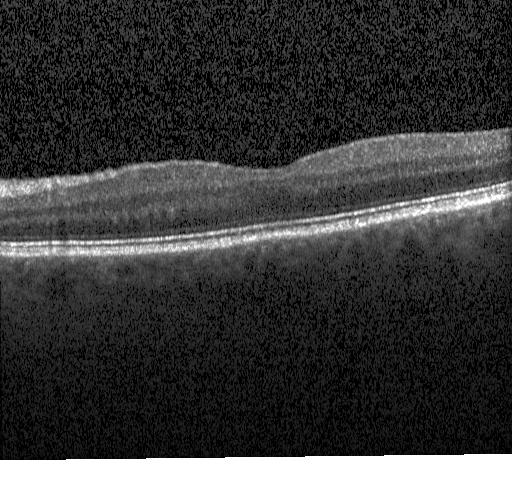
Assessment: no choroidal neovascularization, diabetic macular edema, or drusen.